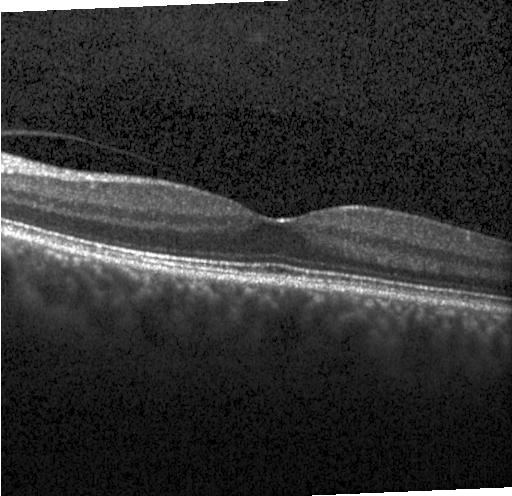
Centered on the fovea · instrument: Heidelberg Spectralis · spectral-domain optical coherence tomography · retinal OCT cross-section — Assessment: no CNV, no DME, and no drusen.